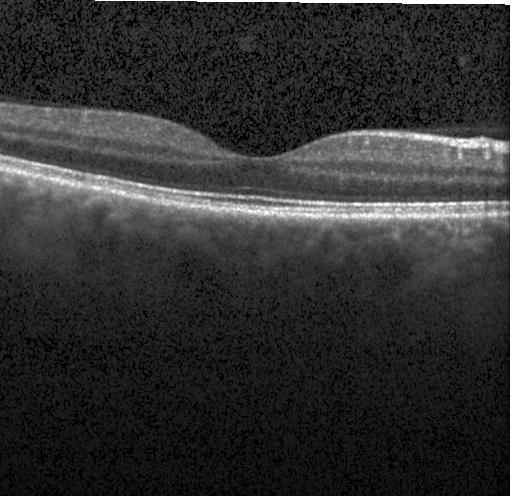

OCT B-scan showing no CNV, DME, or drusen.